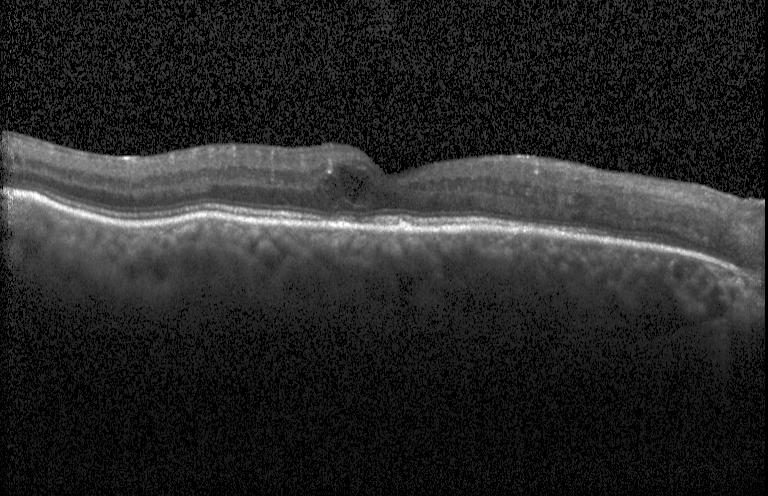 OCT scan showing diabetic macular edema.